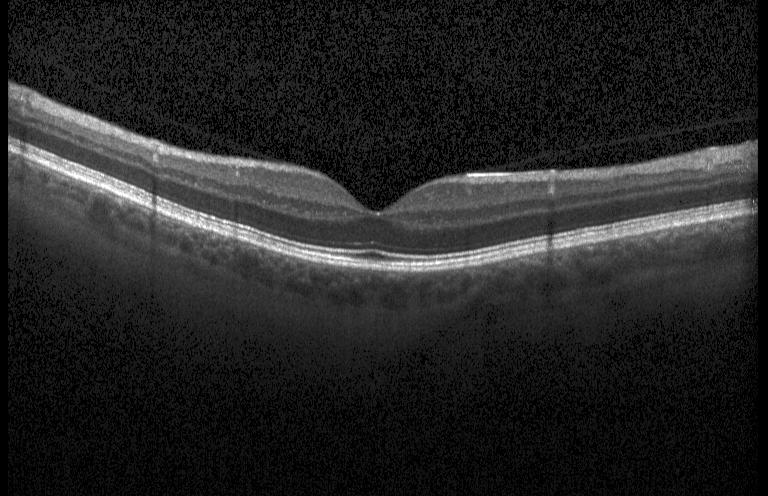 Retinal OCT cross-section · spectral-domain OCT.
Impression: no CNV, DME, or drusen.